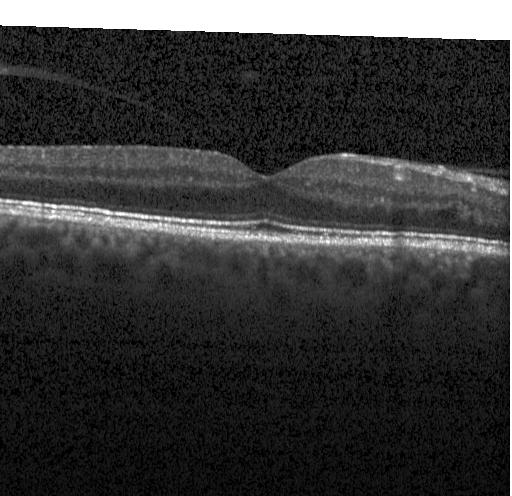

OCT B-scan. Finding: no evidence of choroidal neovascularization, diabetic macular edema, or drusen.